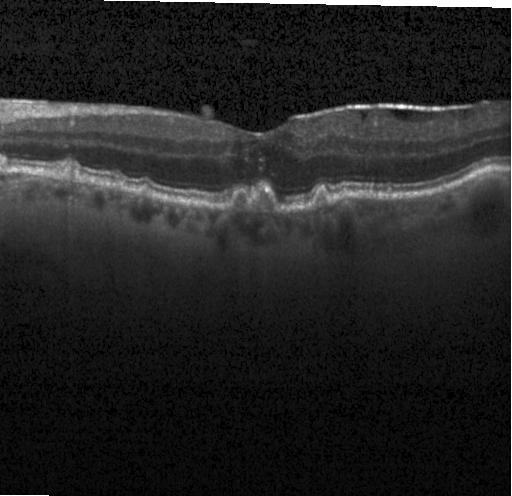
Centered on the fovea; optical coherence tomography scan. Diagnosis: multiple drusen.